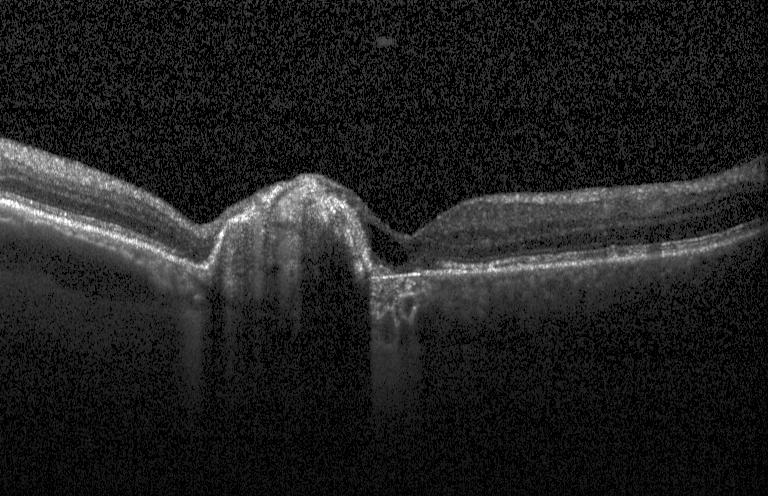 Optical coherence tomography B-scan. Diagnosis: CNV.